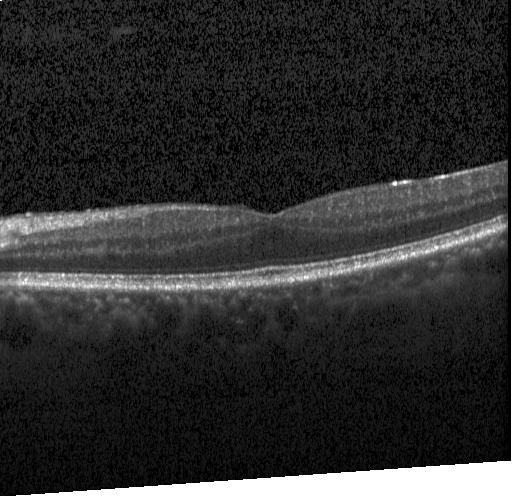
Instrument: Heidelberg Spectralis. OCT line scan — Finding: no CNV, DME, or drusen.